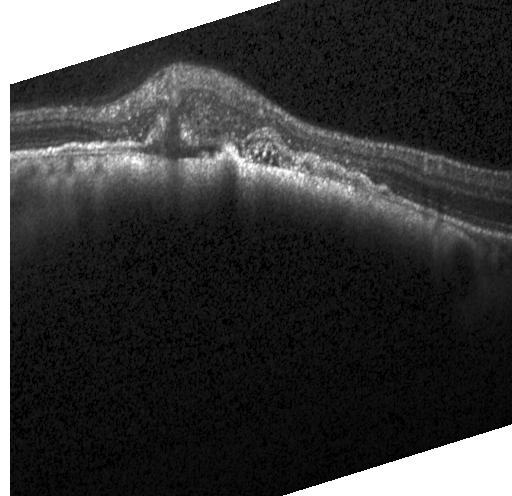
Impression: choroidal neovascularization.